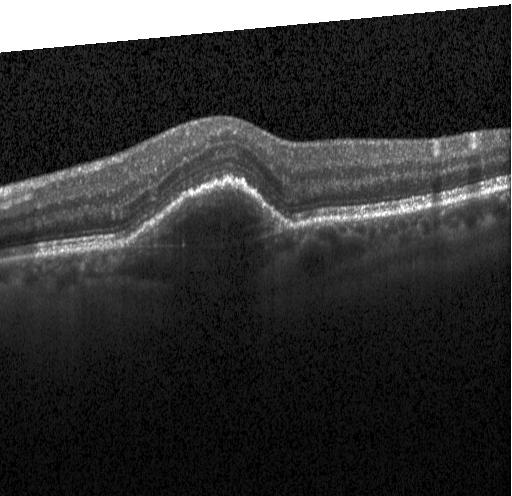 Horizontal scan through the fovea · optical coherence tomography B-scan · SD-OCT — Diagnosis: a choroidal neovascular membrane.